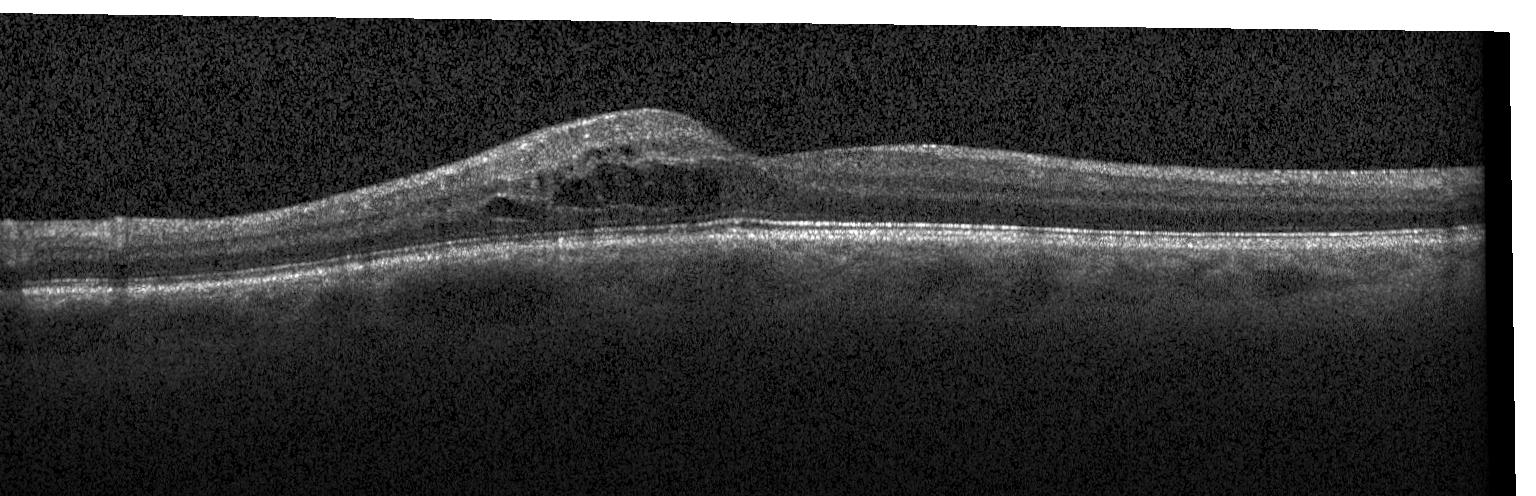 Diagnosis: DME.